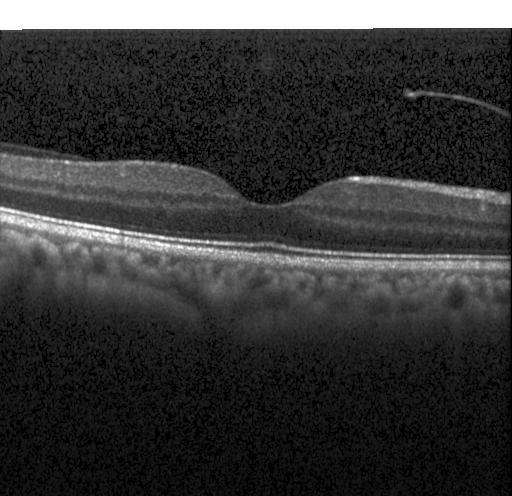

OCT finding: neither CNV, DME, nor drusen.